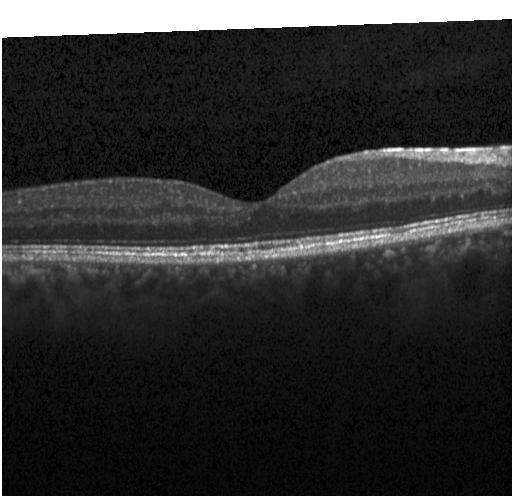 This B-scan demonstrates no evidence of CNV, DME, or drusen.